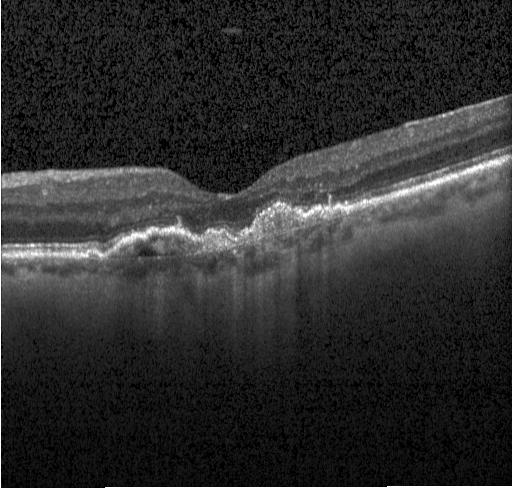
Retinal OCT cross-section · spectral-domain optical coherence tomography — OCT finding: a choroidal neovascular membrane.